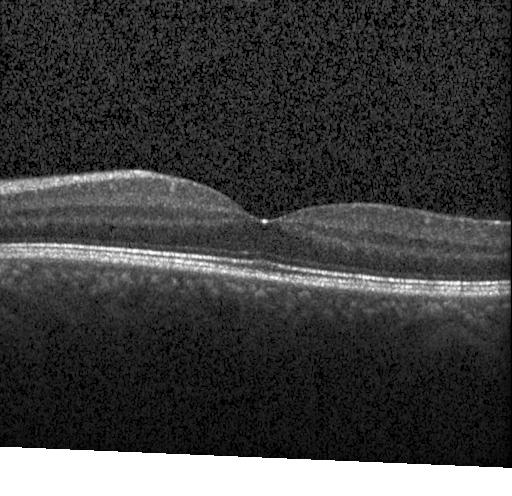
OCT finding: neither choroidal neovascularization, diabetic macular edema, nor drusen.